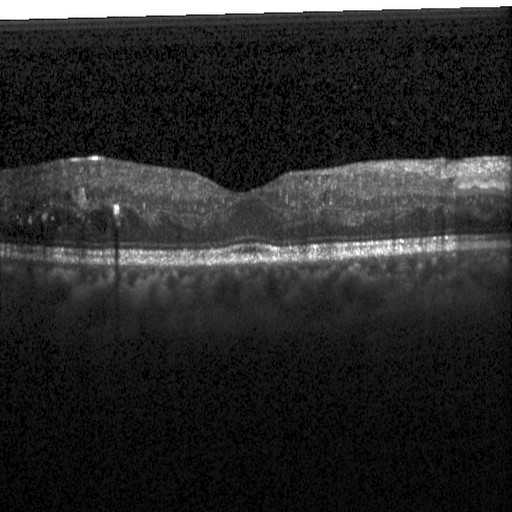 OCT B-scan showing DME.